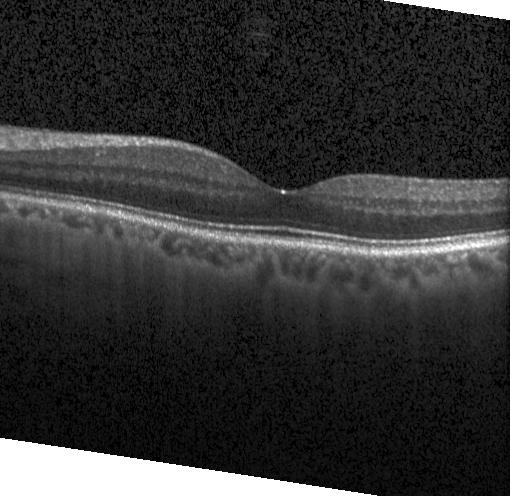

OCT B-scan
Impression: no choroidal neovascularization, diabetic macular edema, or drusen.